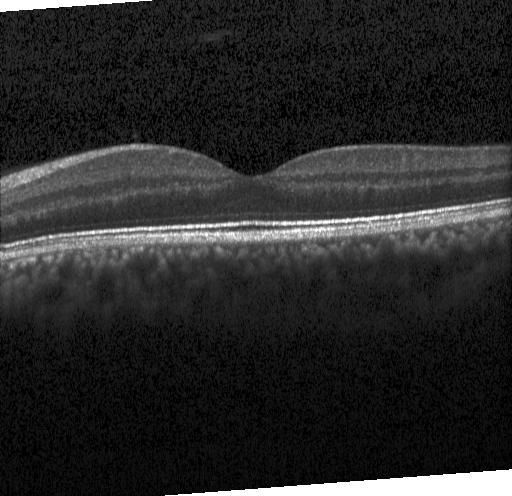

Finding: no evidence of choroidal neovascularization, diabetic macular edema, or drusen.